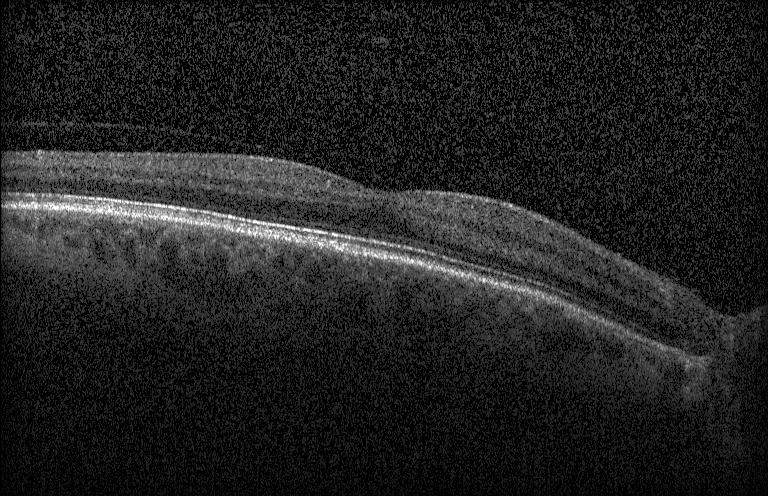 Optical coherence tomography B-scan
The scan shows no evidence of CNV, DME, or drusen.